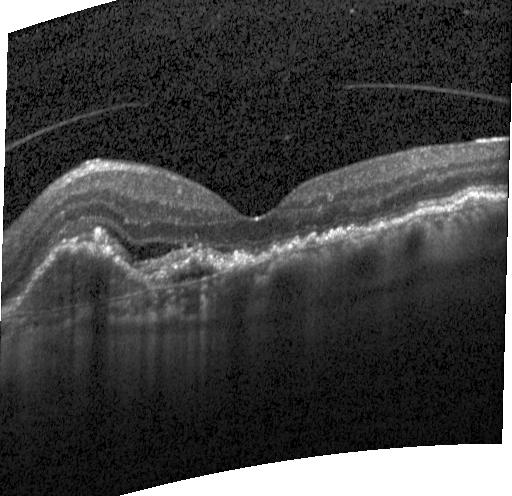 The scan shows a choroidal neovascular membrane.